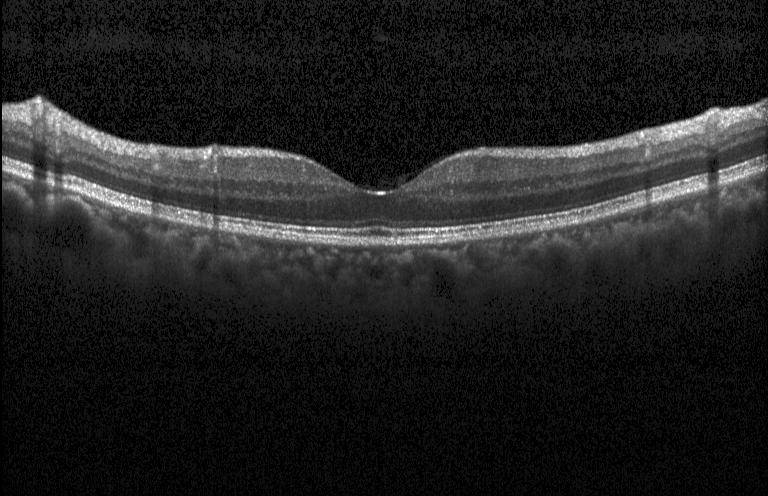

Diagnosis: neither choroidal neovascularization, diabetic macular edema, nor drusen.